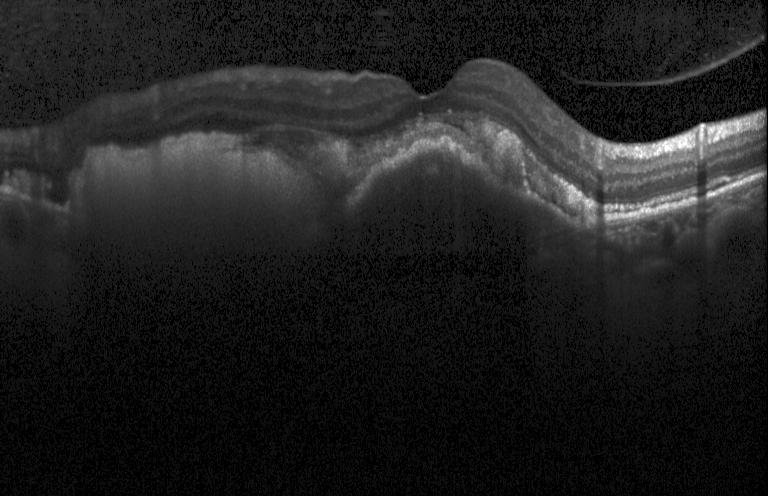
Retinal OCT cross-section; fovea-centered.
Macular OCT: a choroidal neovascular membrane.